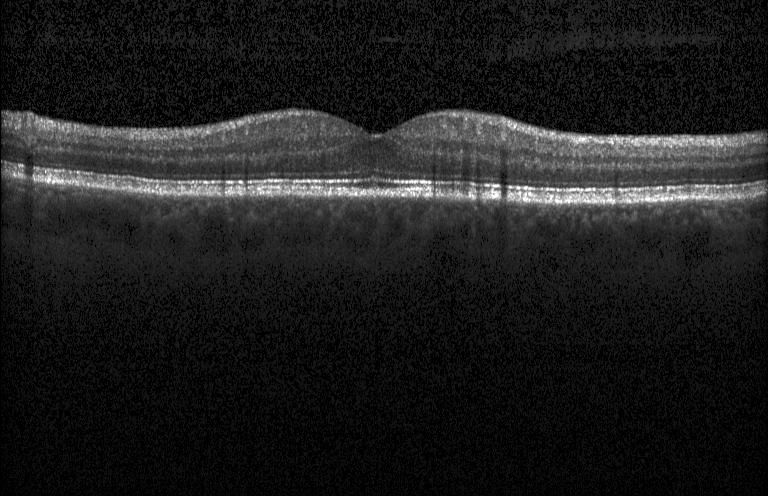 Heidelberg Spectralis · retinal OCT cross-section — Impression: no choroidal neovascularization, diabetic macular edema, or drusen.